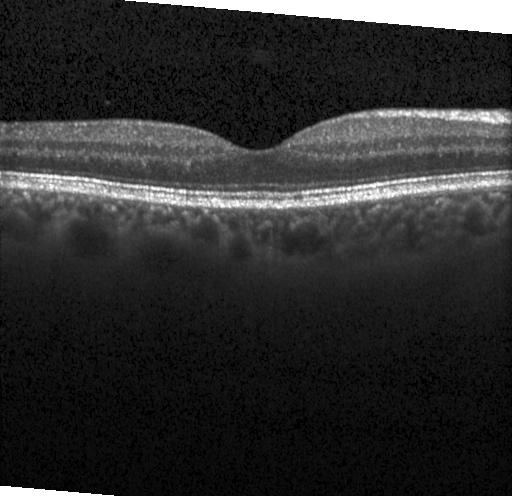

Macular scan. SD-OCT. Heidelberg Spectralis OCT system. Retinal OCT cross-section
Assessment: no choroidal neovascularization, no diabetic macular edema, and no drusen.